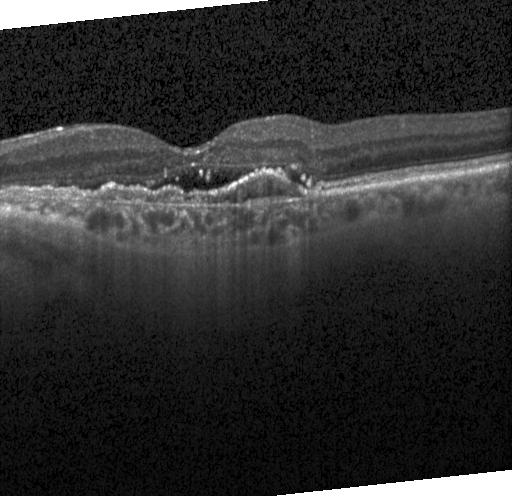
This B-scan demonstrates a choroidal neovascular membrane.